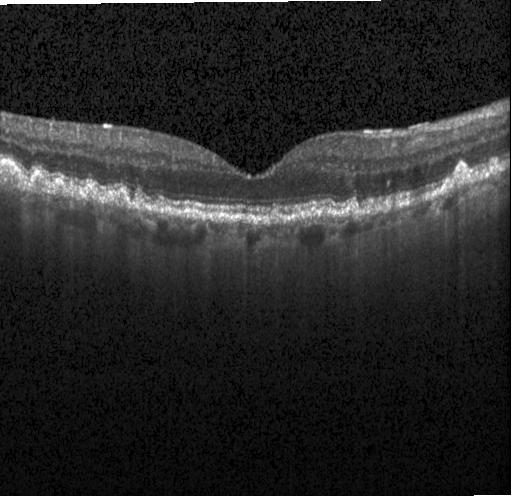

Centered on the fovea, OCT B-scan, SD-OCT. Assessment: sub-RPE drusenoid deposits.